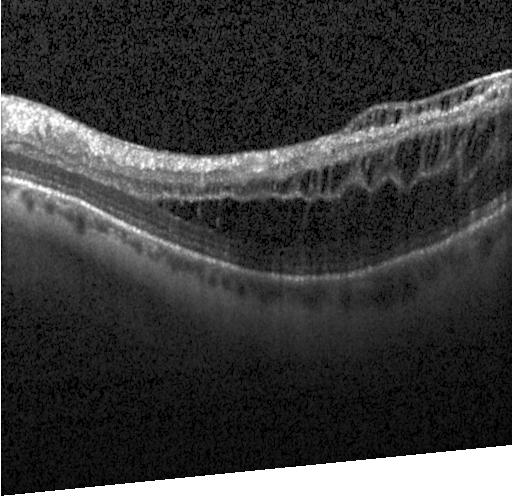 The scan shows DME.